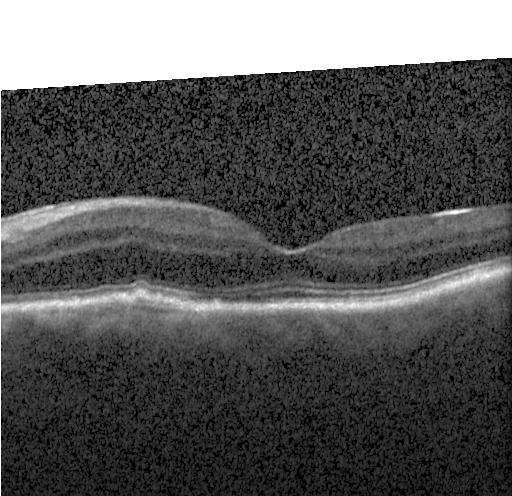 Finding: multiple drusen.